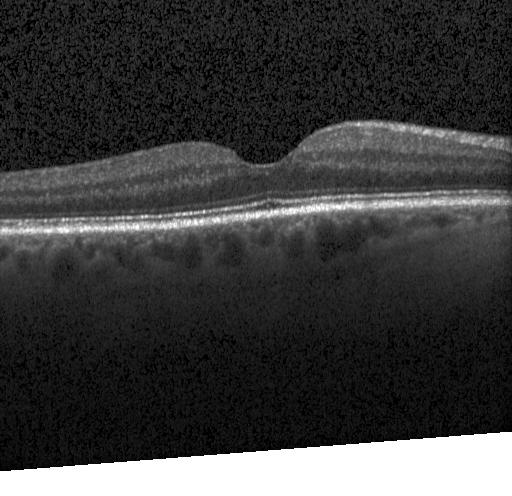

OCT finding: no choroidal neovascularization, diabetic macular edema, or drusen.